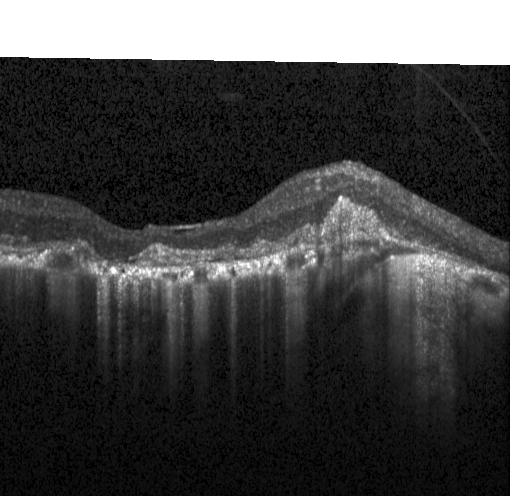

Centered on the fovea; spectral-domain optical coherence tomography; retinal OCT cross-section
Dx: a choroidal neovascular membrane.